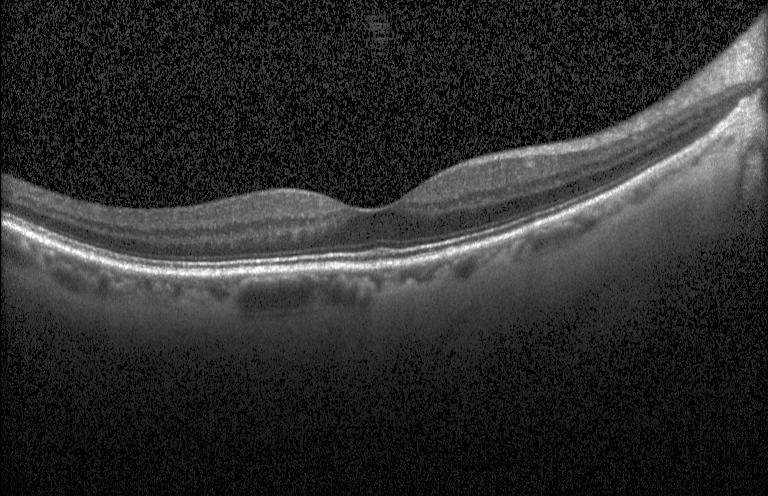
Spectral-domain optical coherence tomography; optical coherence tomography scan
Finding: no choroidal neovascularization, diabetic macular edema, or drusen.